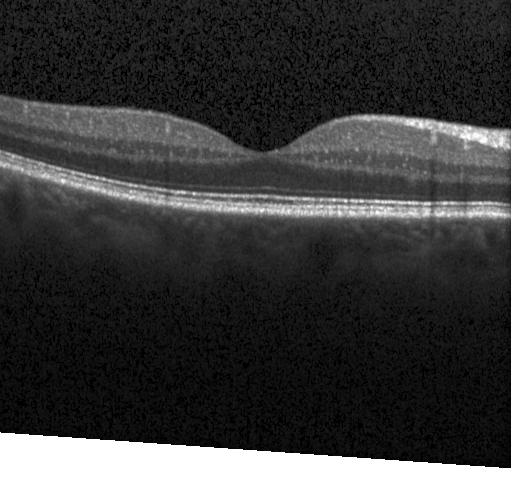 No choroidal neovascularization, no diabetic macular edema, and no drusen.